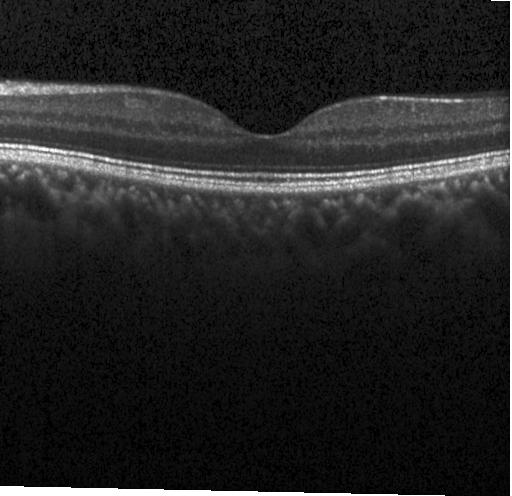
Heidelberg Spectralis OCT system, retinal OCT cross-section, through the macula. Finding: neither choroidal neovascularization, diabetic macular edema, nor drusen.